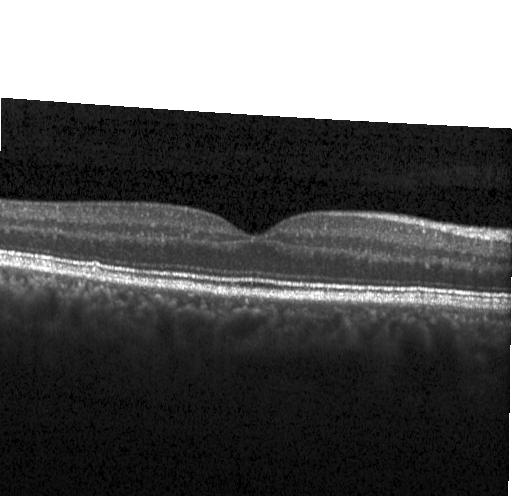
Impression: no evidence of CNV, DME, or drusen.